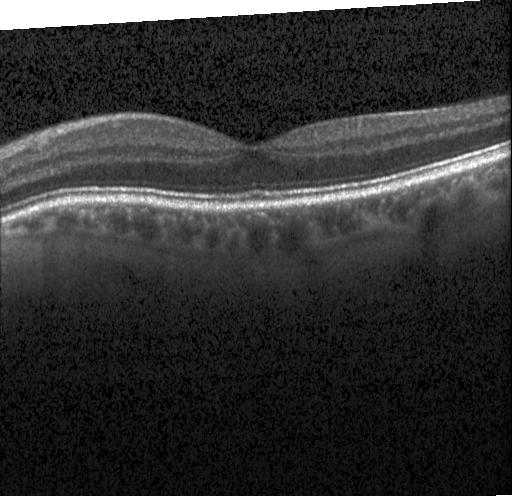 Optical coherence tomography scan; SD-OCT.
Diagnosis: no evidence of choroidal neovascularization, diabetic macular edema, or drusen.